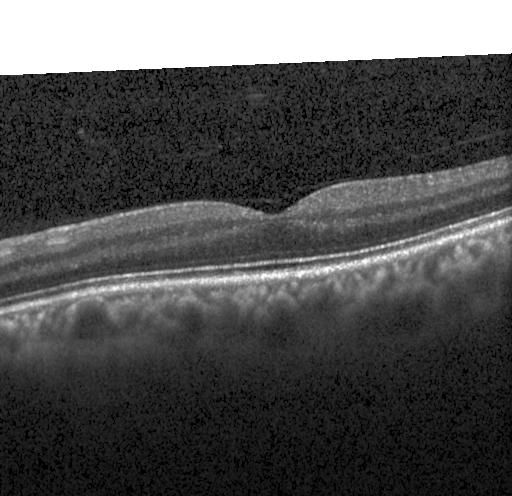
Retinal OCT cross-section. Instrument: Heidelberg Spectralis. This B-scan demonstrates no choroidal neovascularization, diabetic macular edema, or drusen.